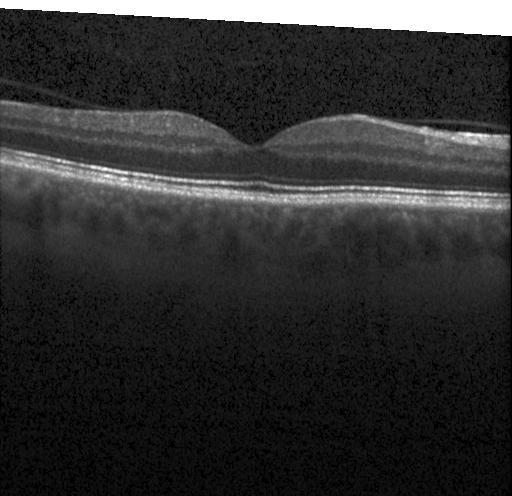 Optical coherence tomography B-scan. Macular OCT: no CNV, no DME, and no drusen.